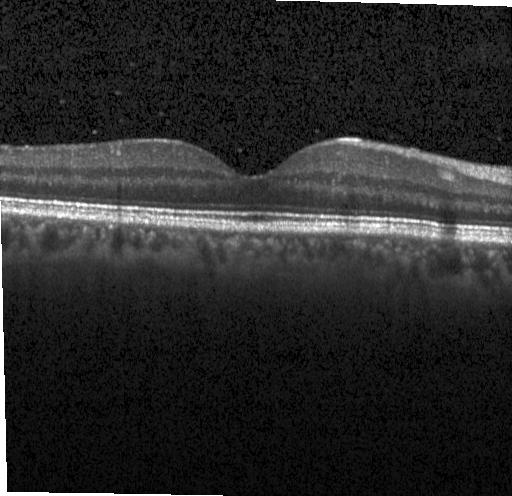
OCT line scan.
Diagnosis: no choroidal neovascularization, diabetic macular edema, or drusen.